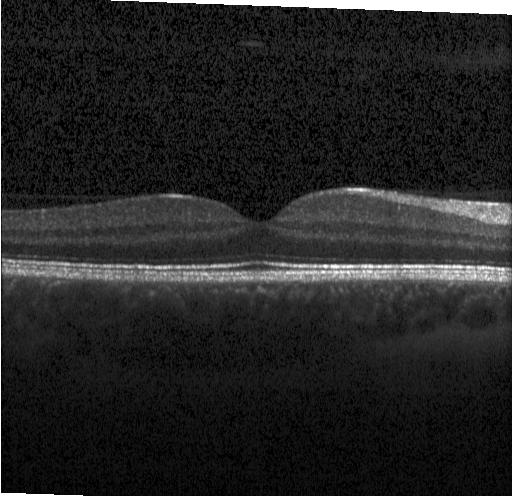

OCT B-scan showing no choroidal neovascularization, no diabetic macular edema, and no drusen.